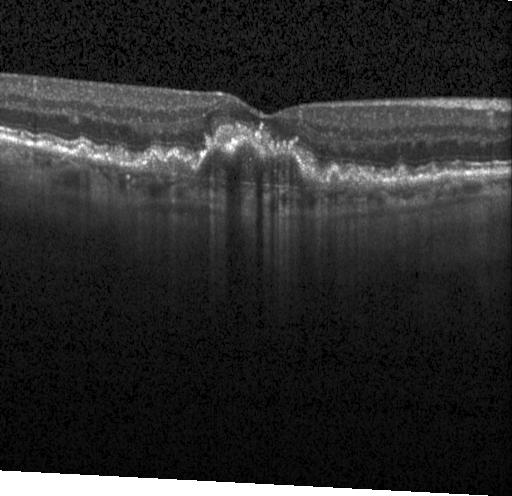 SD-OCT, macular scan, OCT line scan.
Diagnosis: a choroidal neovascular membrane.